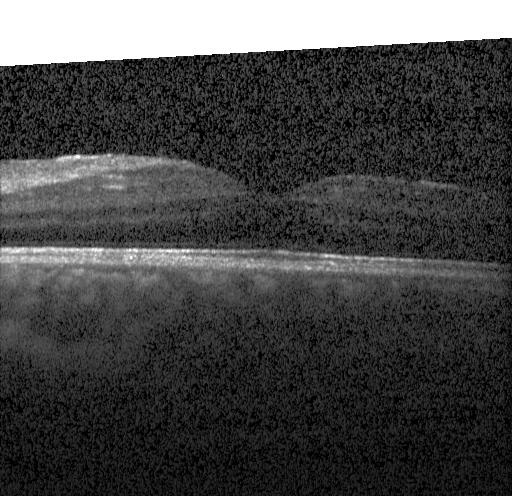

Diagnosis: no choroidal neovascularization, diabetic macular edema, or drusen.